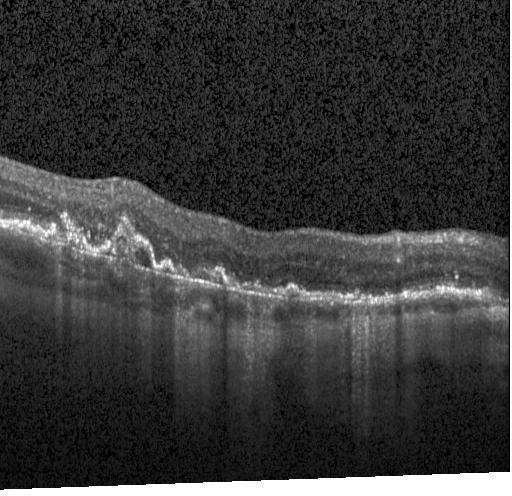 Retinal OCT B-scan
This B-scan demonstrates a choroidal neovascular membrane.